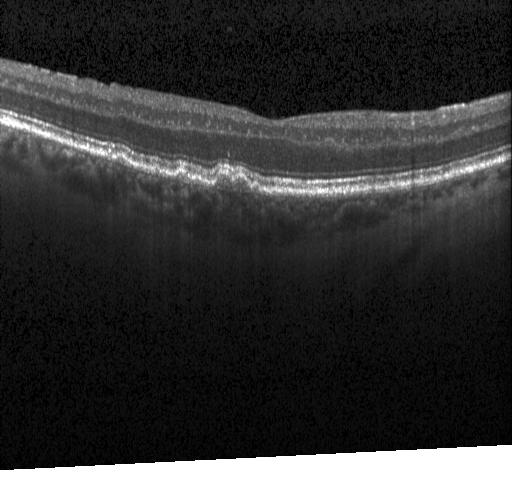
OCT line scan.
Diagnosis: multiple drusen.